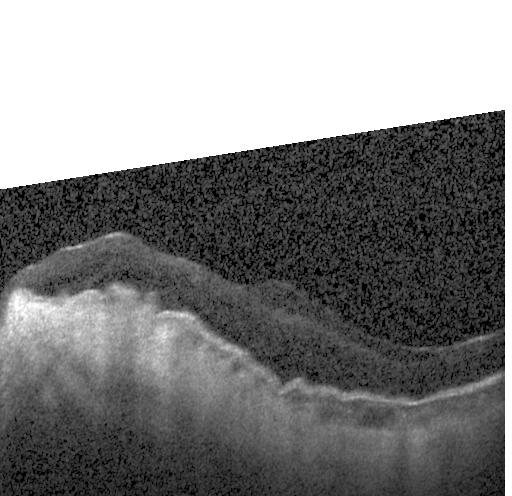
This B-scan demonstrates a choroidal neovascular membrane.